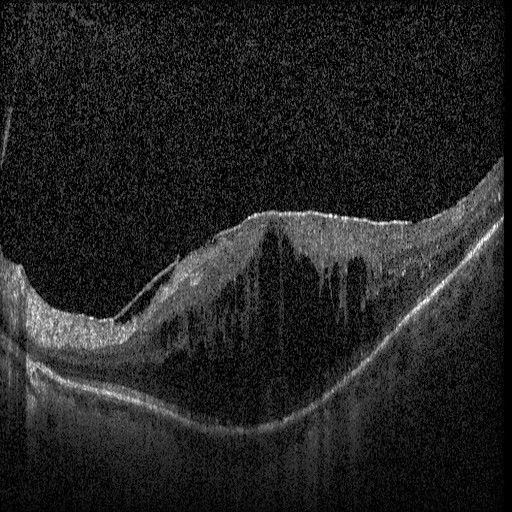 Through the macula; optical coherence tomography B-scan.
Impression: diabetic macular edema (DME).